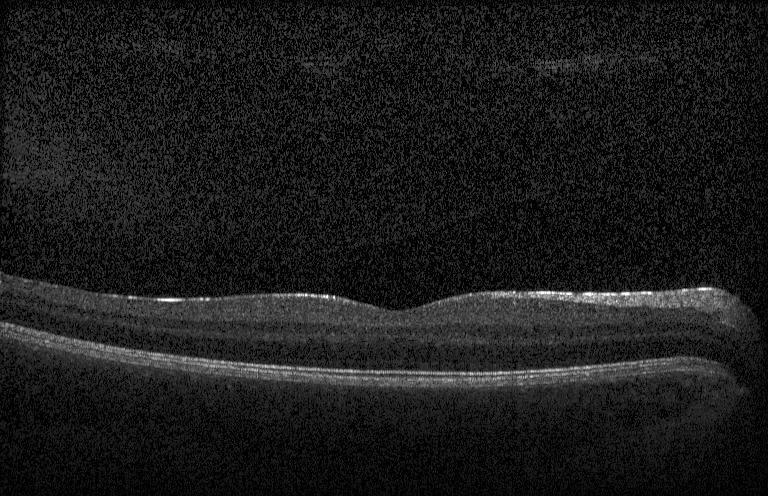

OCT finding: no CNV, no DME, and no drusen.